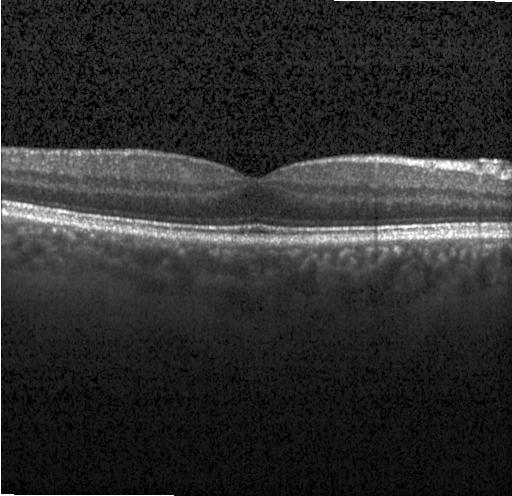

Heidelberg Spectralis. Optical coherence tomography B-scan. Centered on the fovea. The scan shows neither choroidal neovascularization, diabetic macular edema, nor drusen.